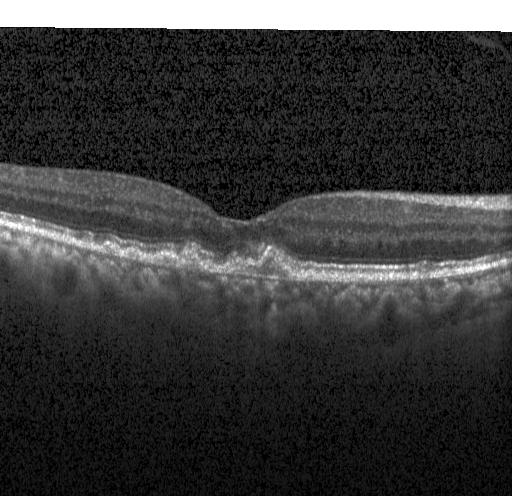
Macular OCT demonstrating a choroidal neovascular membrane.